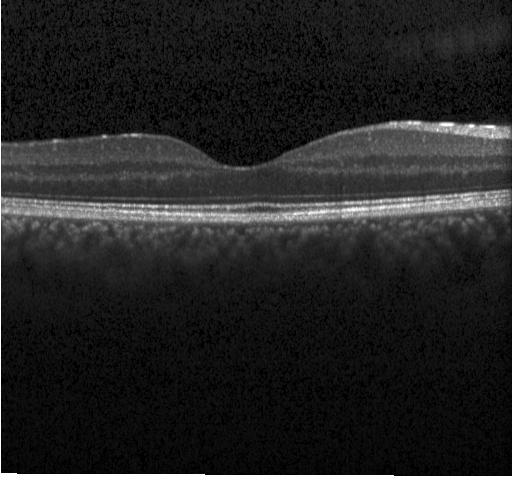 Fovea-centered · optical coherence tomography scan · instrument: Heidelberg Spectralis.
Impression: no choroidal neovascularization, no diabetic macular edema, and no drusen.